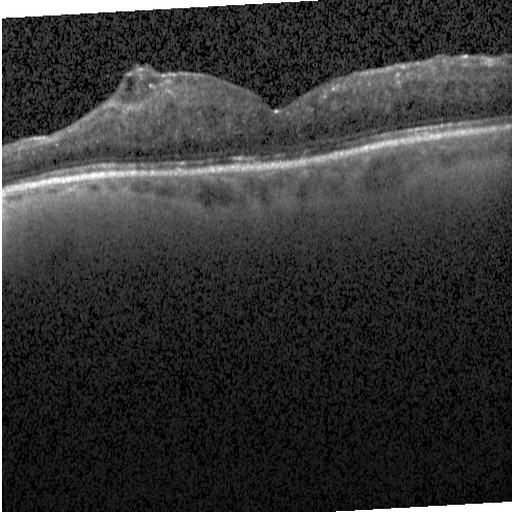

Macular scan; spectral-domain optical coherence tomography; retinal OCT cross-section
Diagnosis: diabetic macular edema.